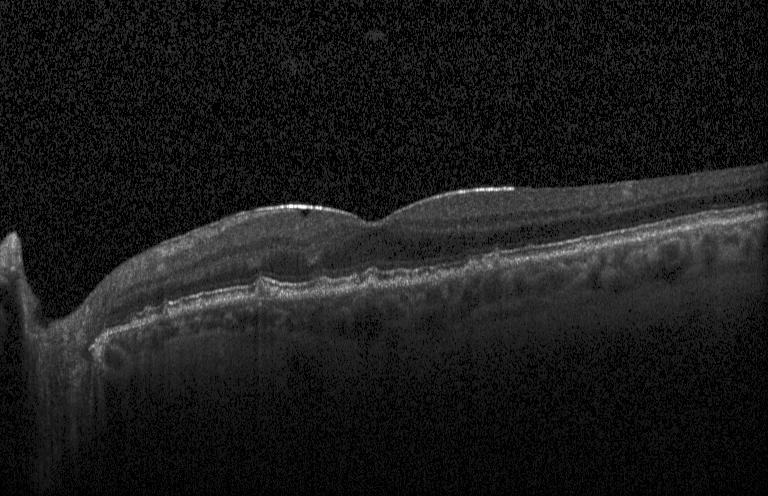

Diagnosis: drusen.